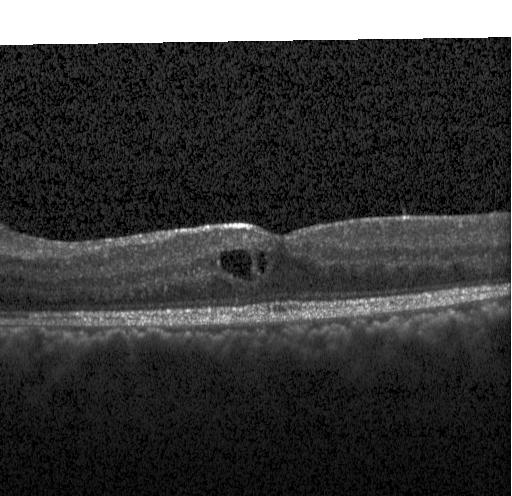
OCT line scan, through the macula, acquired on a Heidelberg Spectralis, spectral-domain optical coherence tomography
Diabetic macular edema (DME).